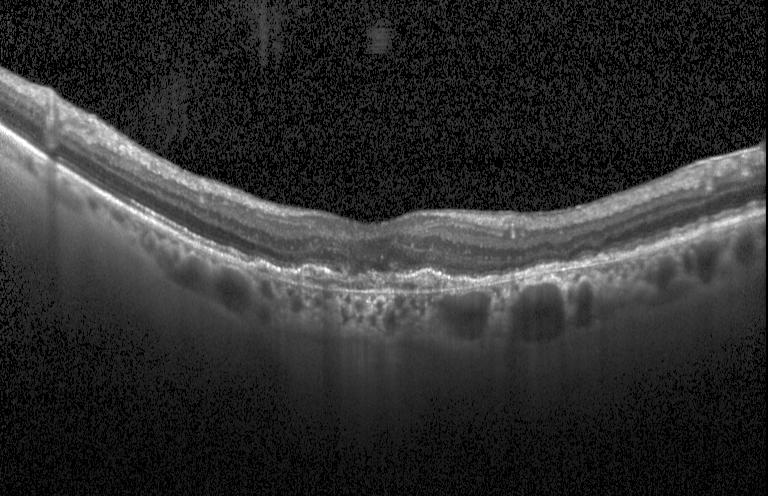
Diagnosis: a choroidal neovascular membrane.